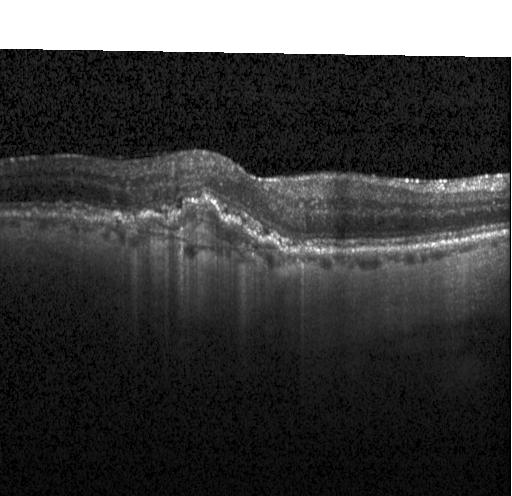 Impression: choroidal neovascularization (CNV).